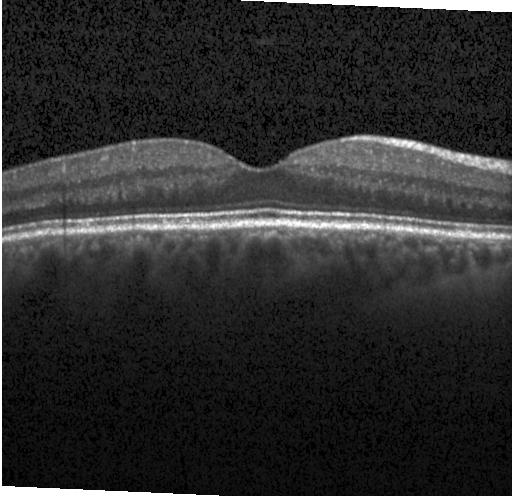

Spectral-domain OCT B-scan: no CNV, no DME, and no drusen.